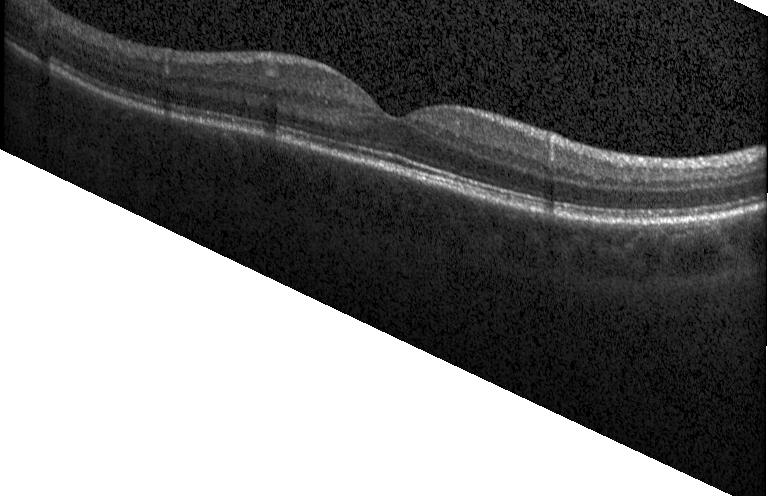 Optical coherence tomography scan. The scan shows no evidence of CNV, DME, or drusen.